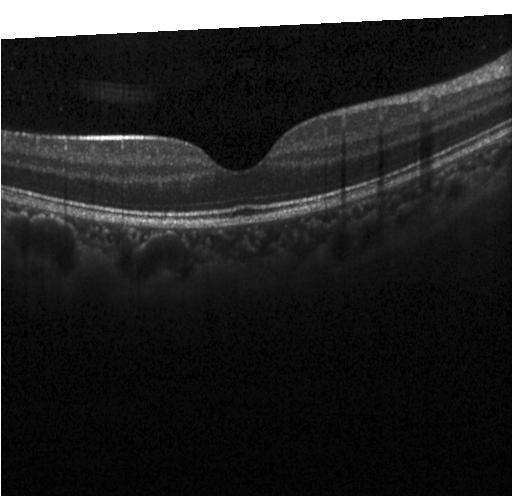
SD-OCT, acquired on a Heidelberg Spectralis, fovea-centered, optical coherence tomography scan. Finding: no evidence of CNV, DME, or drusen.